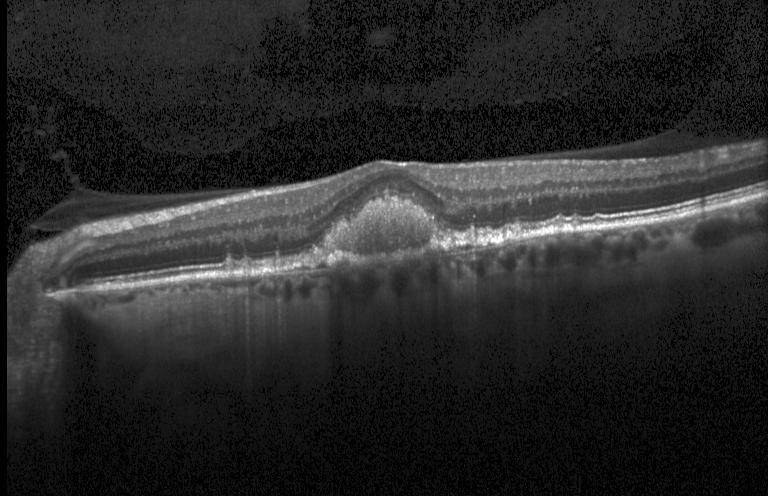 Retinal OCT B-scan.
Diagnosis: CNV.